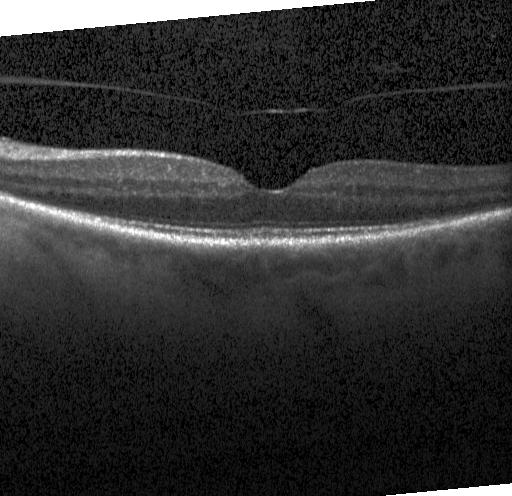 OCT B-scan.
Diagnosis: neither choroidal neovascularization, diabetic macular edema, nor drusen.